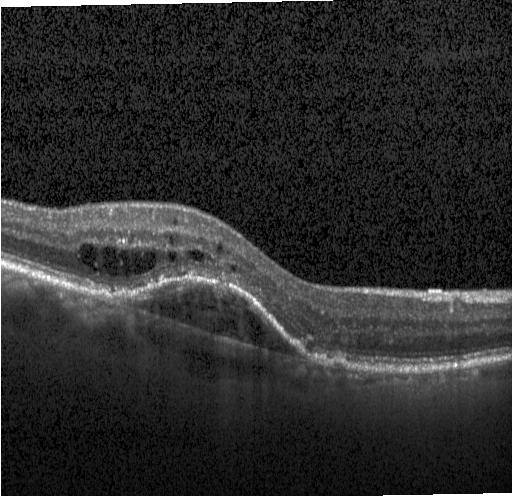 OCT B-scan. Spectral-domain OCT. Acquired on a Heidelberg Spectralis.
Impression: a choroidal neovascular membrane.